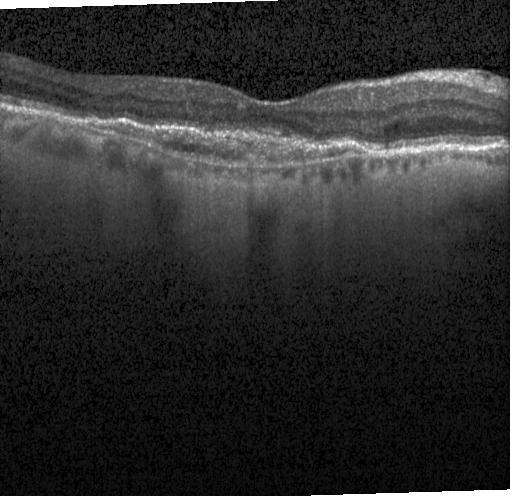

Finding: a choroidal neovascular membrane.